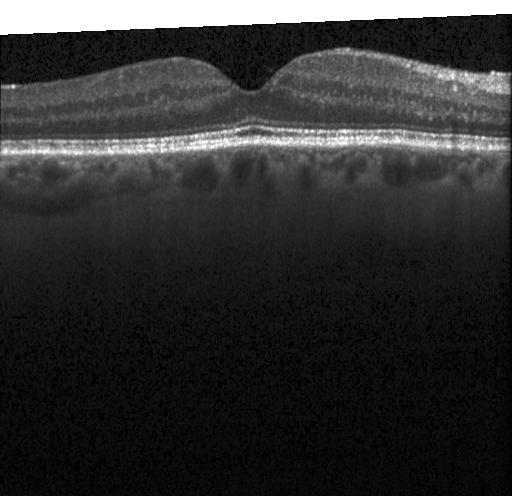
OCT B-scan — Impression: no CNV, DME, or drusen.